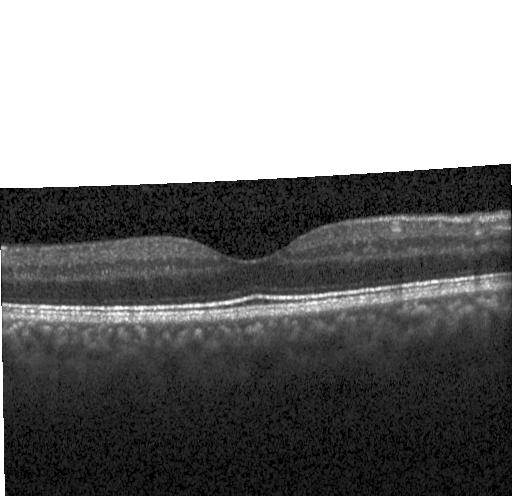

Diagnosis: no choroidal neovascularization, diabetic macular edema, or drusen.